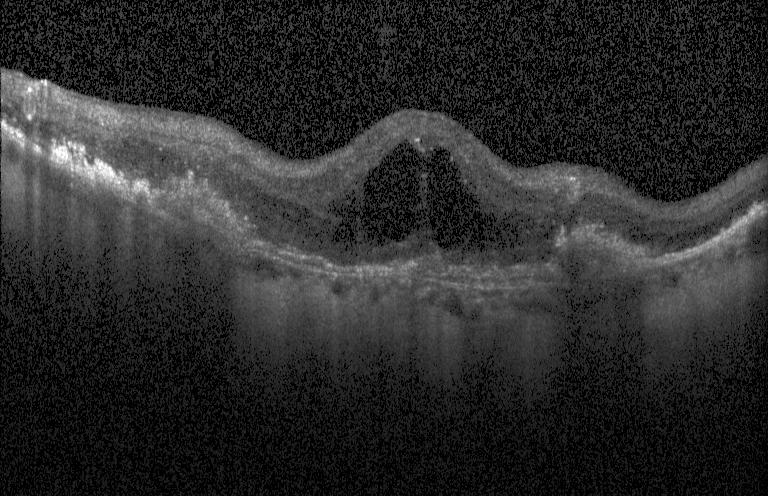 Fovea-centered; retinal OCT cross-section
Macular OCT: a choroidal neovascular membrane.